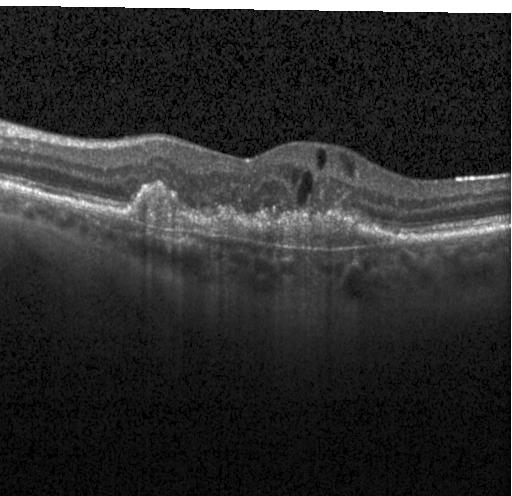
Macular scan. Optical coherence tomography scan. Acquired on a Heidelberg Spectralis. Impression: a choroidal neovascular membrane.